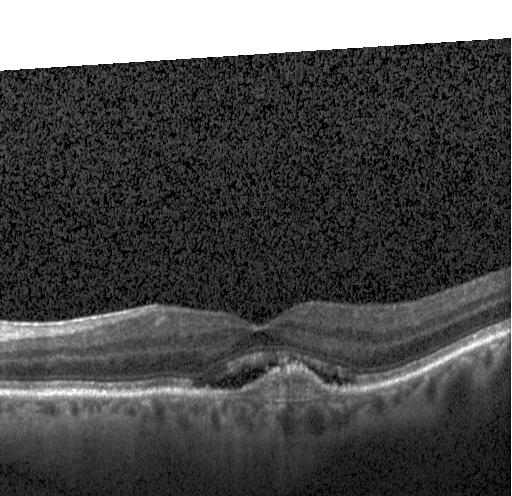

OCT line scan
Dx: choroidal neovascularization (CNV).